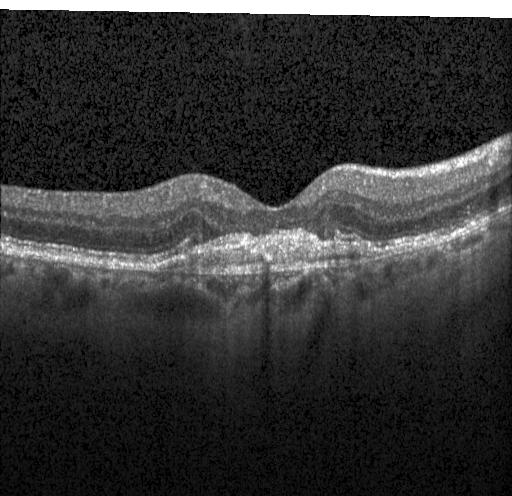 Choroidal neovascularization.